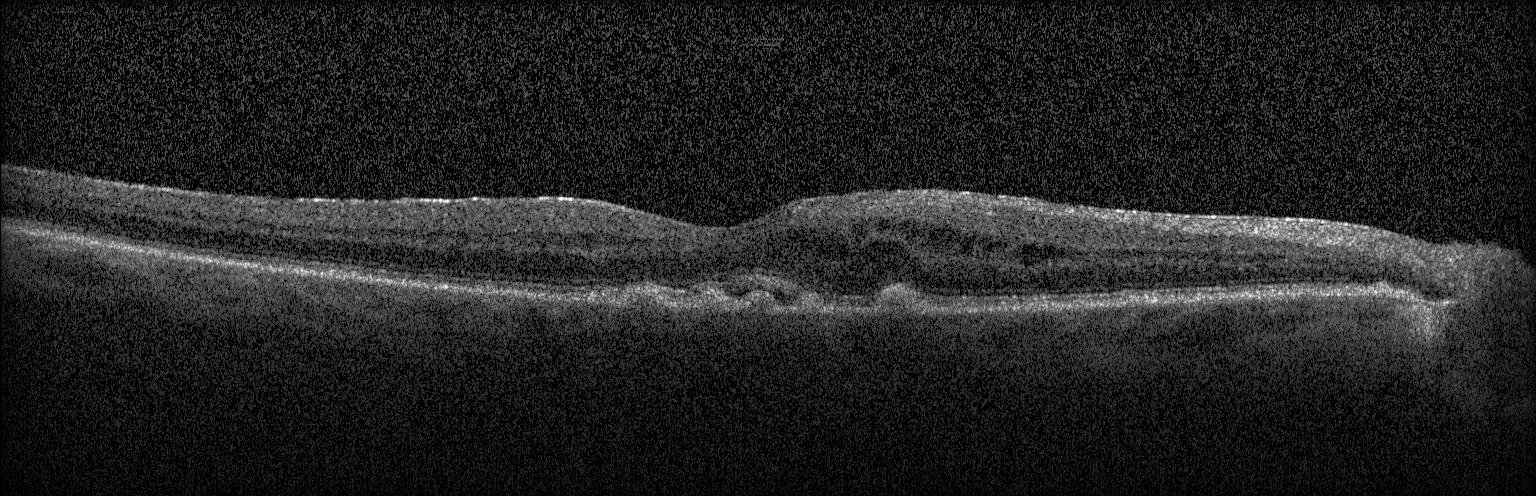

Spectral-domain OCT B-scan: choroidal neovascularization (CNV).